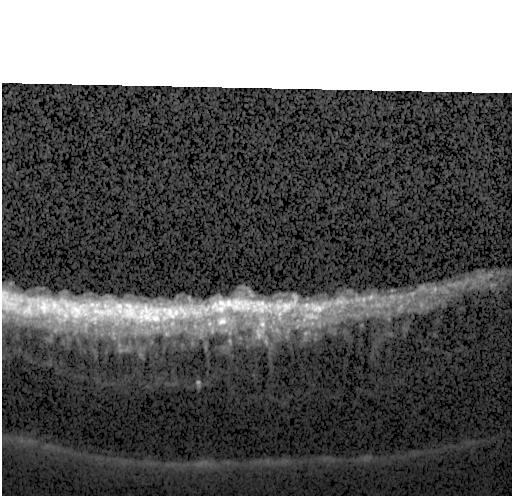 SD-OCT · OCT line scan · through the macula · Heidelberg Spectralis.
Macular OCT: diabetic macular edema.